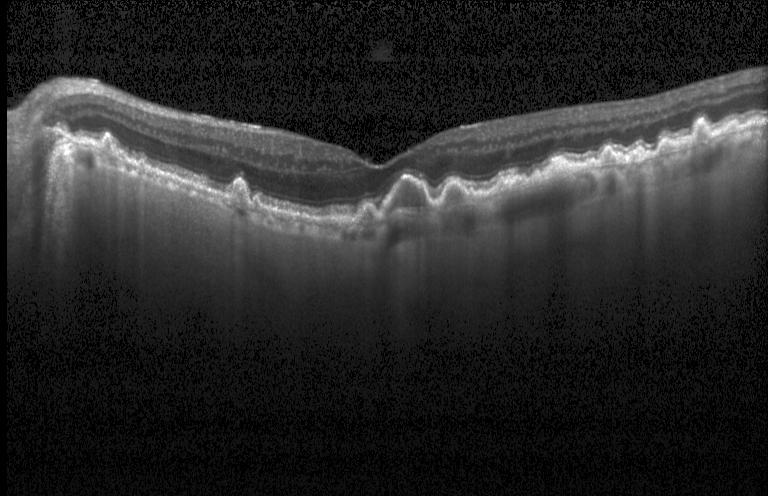 Heidelberg Spectralis. Spectral-domain optical coherence tomography. Fovea-centered. Optical coherence tomography scan
OCT finding: multiple drusen.